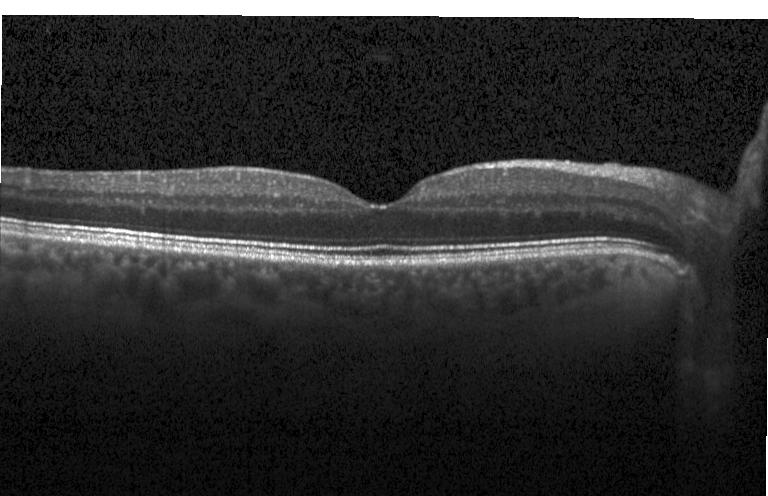
SD-OCT · retinal OCT B-scan · Heidelberg Spectralis · macular scan
OCT finding: no choroidal neovascularization, no diabetic macular edema, and no drusen.